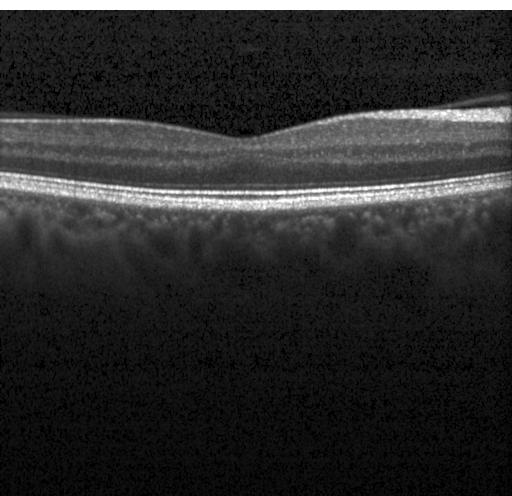
Macular scan, OCT line scan, instrument: Heidelberg Spectralis, spectral-domain OCT — Finding: no evidence of choroidal neovascularization, diabetic macular edema, or drusen.